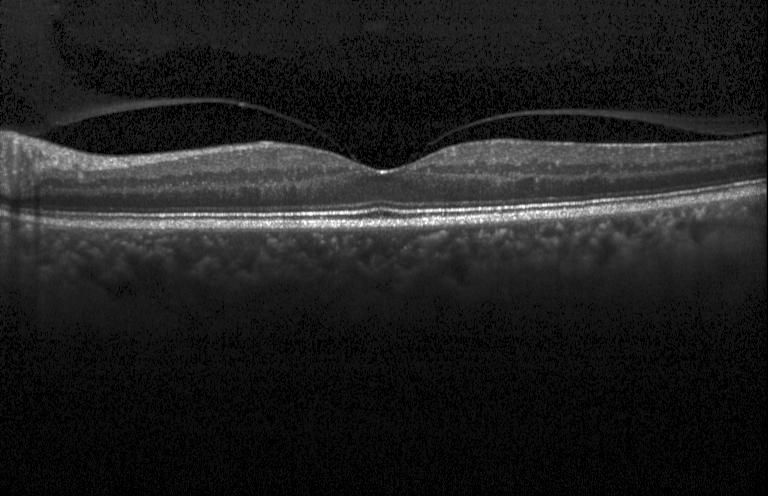
Diagnosis: no evidence of choroidal neovascularization, diabetic macular edema, or drusen.